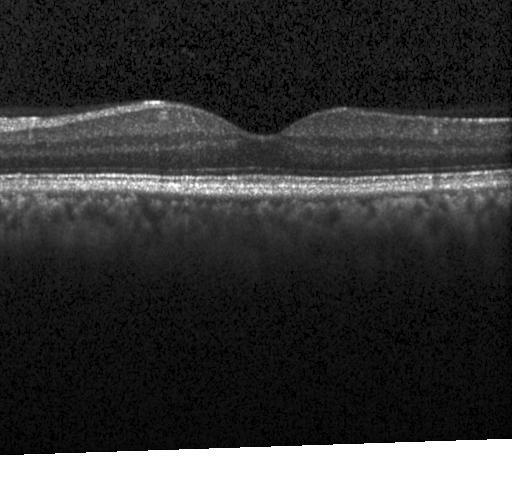
Impression: no CNV, no DME, and no drusen.